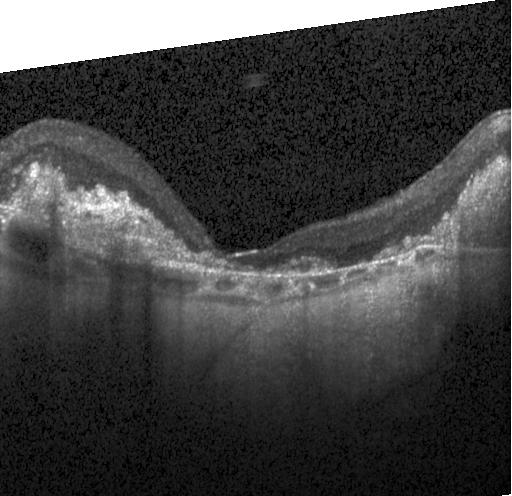
Acquired on a Heidelberg Spectralis. Spectral-domain OCT. Optical coherence tomography scan.
Impression: choroidal neovascularization.